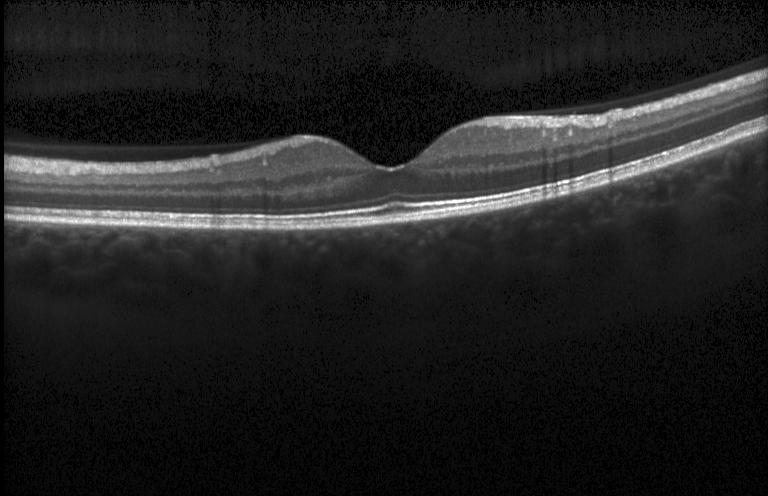

Optical coherence tomography scan · SD-OCT · macular scan.
Impression: no choroidal neovascularization, diabetic macular edema, or drusen.